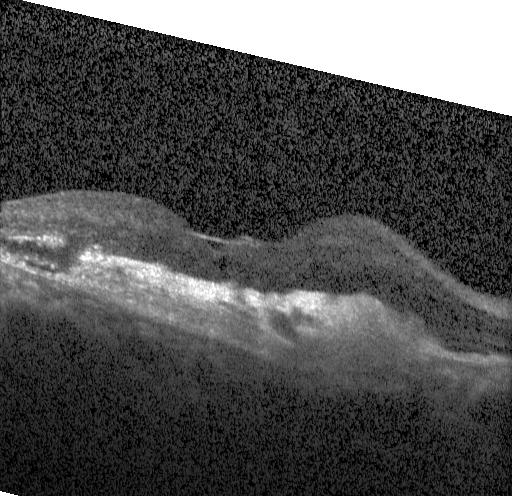

SD-OCT. Macular scan. Retinal OCT B-scan. Acquired on a Heidelberg Spectralis — Assessment: choroidal neovascularization (CNV).